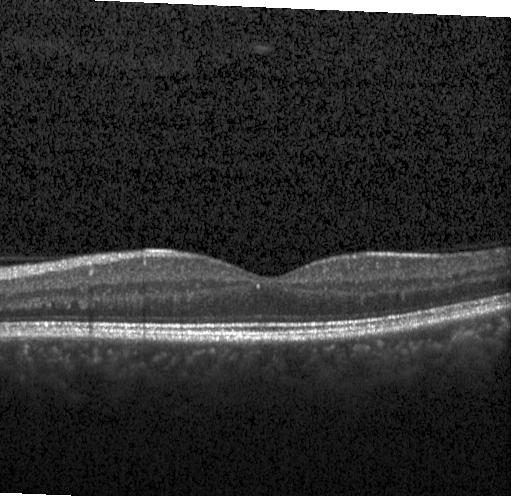 Diagnosis: no CNV, DME, or drusen.